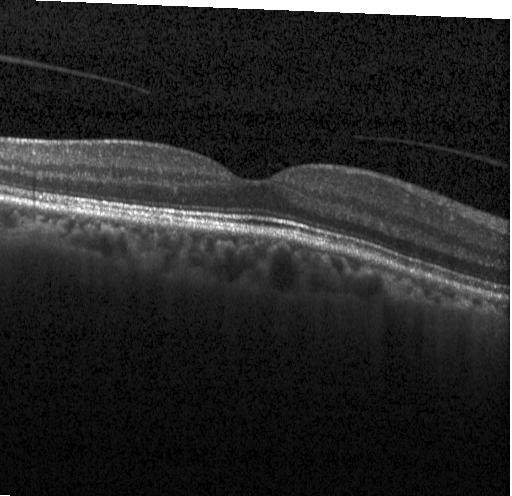

Through the macula · retinal OCT B-scan · spectral-domain optical coherence tomography · acquired on a Heidelberg Spectralis.
This B-scan demonstrates neither choroidal neovascularization, diabetic macular edema, nor drusen.